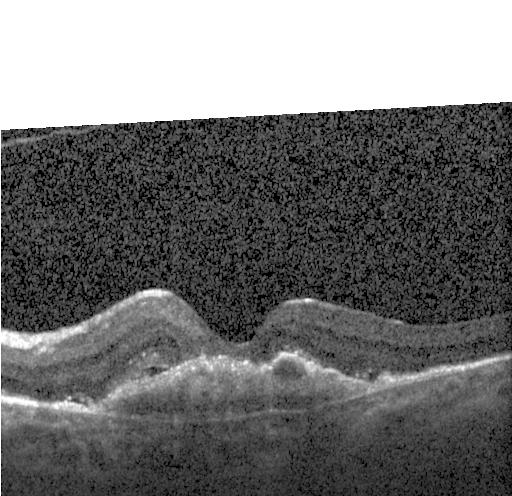

OCT B-scan showing choroidal neovascularization.